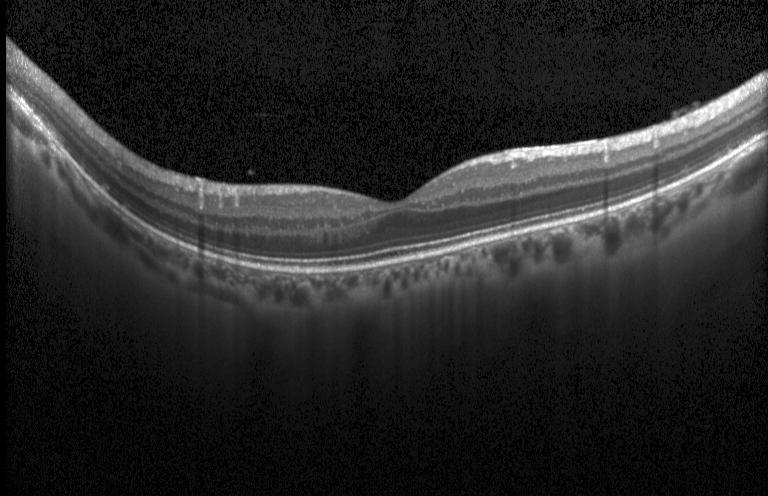

Impression: no CNV, no DME, and no drusen.